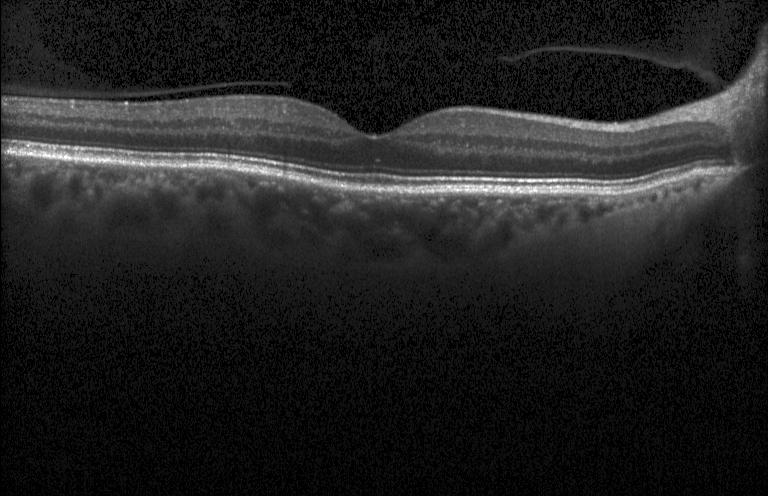

Optical coherence tomography B-scan
Diagnosis: neither CNV, DME, nor drusen.